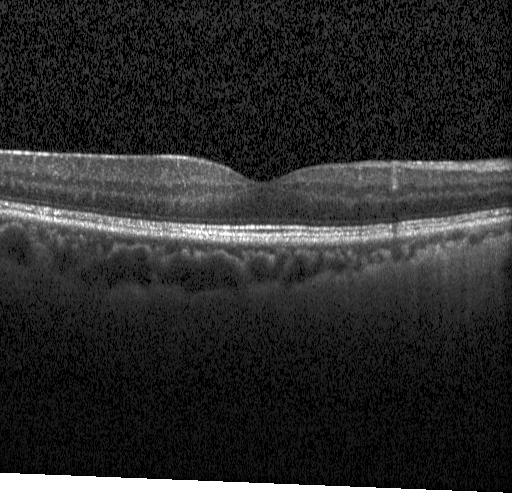 Finding: no choroidal neovascularization, diabetic macular edema, or drusen.